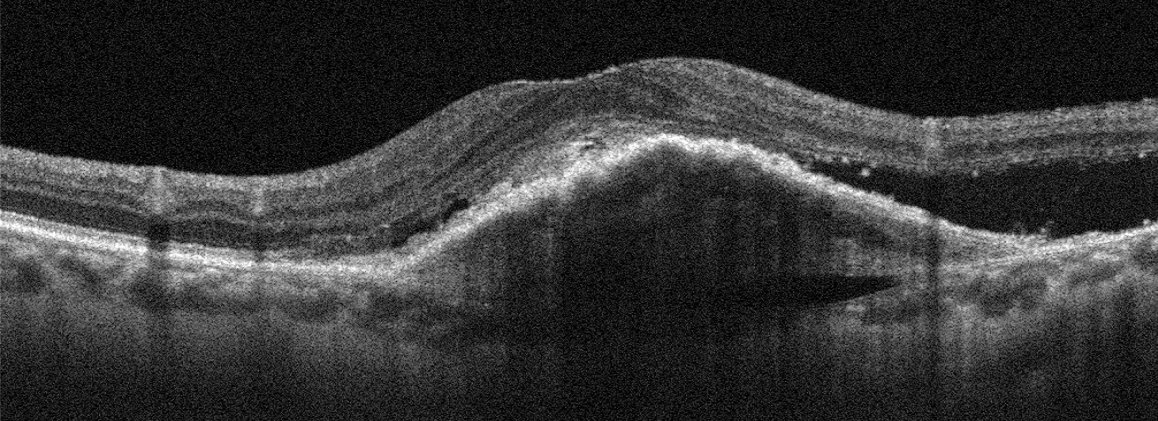 Fovea-centered; retinal OCT B-scan; acquired on an Optovue Avanti RTVue XR. Diagnosis: age-related macular degeneration.